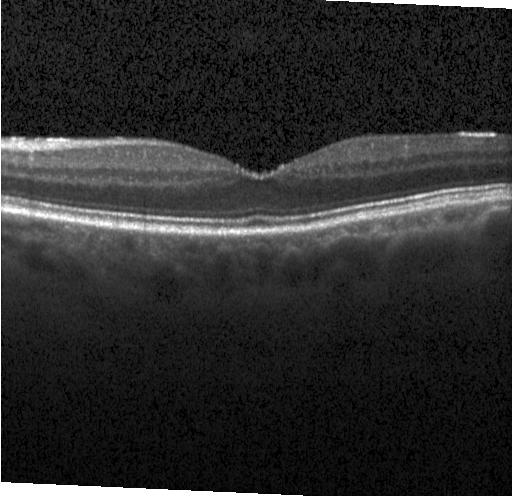 This B-scan demonstrates no choroidal neovascularization, no diabetic macular edema, and no drusen.